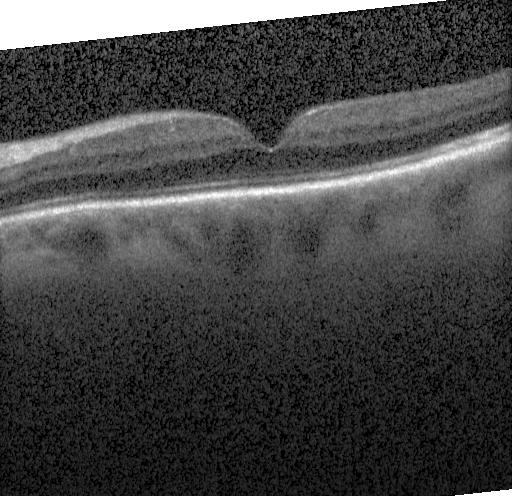

Assessment: no evidence of CNV, DME, or drusen.